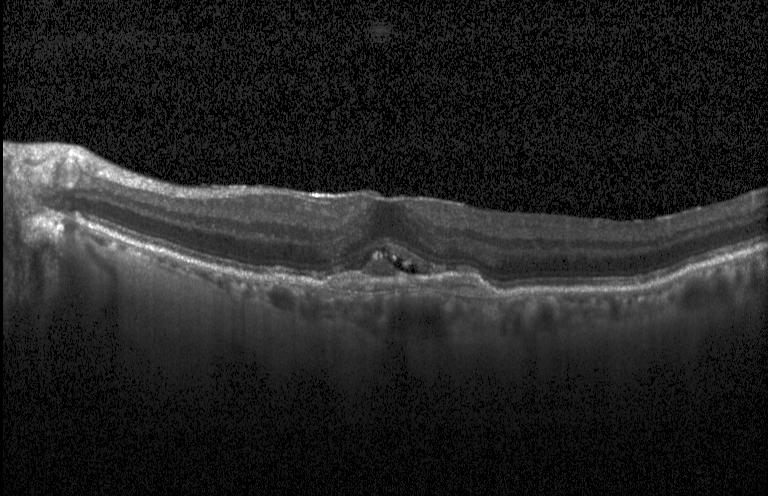

Spectral-domain optical coherence tomography, acquired on a Heidelberg Spectralis, through the macula, optical coherence tomography B-scan. OCT finding: CNV.